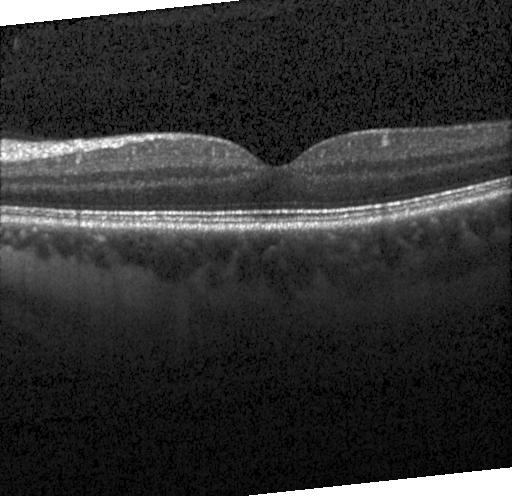 Diagnosis: no CNV, no DME, and no drusen.